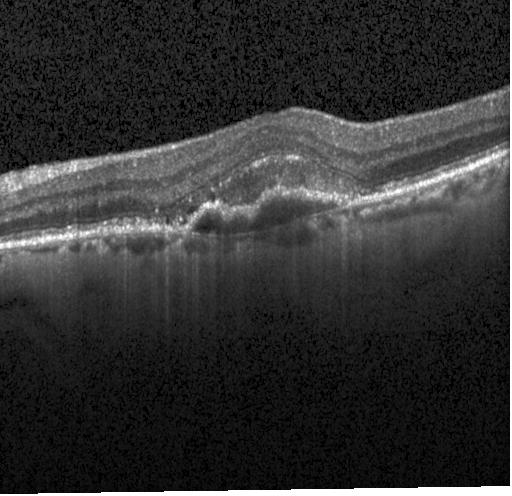
Instrument: Heidelberg Spectralis; spectral-domain optical coherence tomography; OCT B-scan — Dx: a choroidal neovascular membrane.